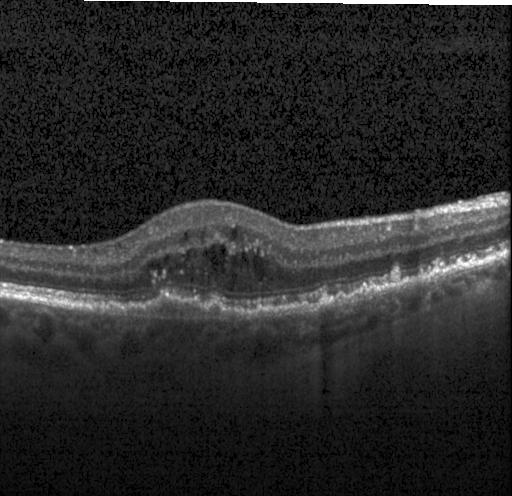 Optical coherence tomography scan
Finding: a choroidal neovascular membrane.